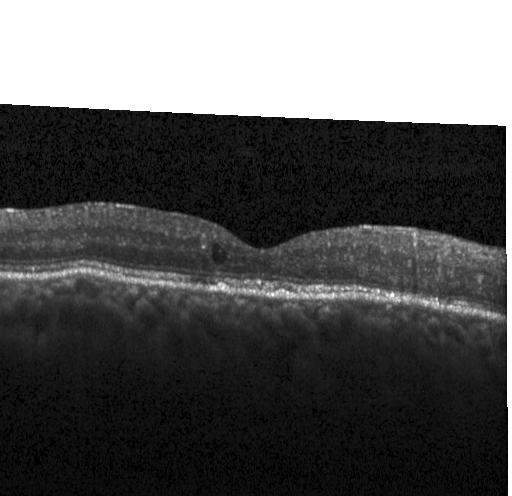 Diagnosis: diabetic macular edema.